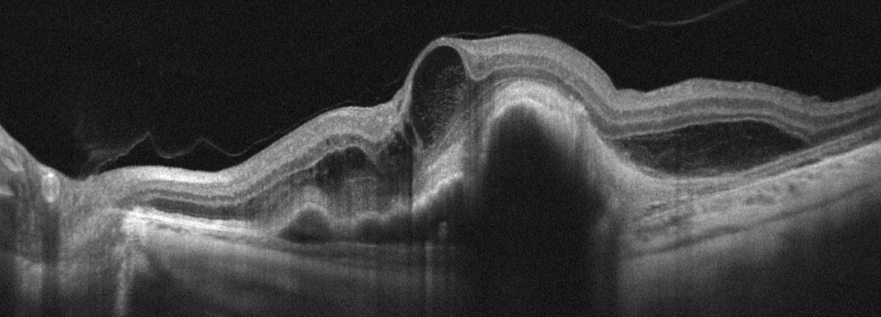 Macular scan; OCT B-scan — Age-related macular degeneration (AMD).